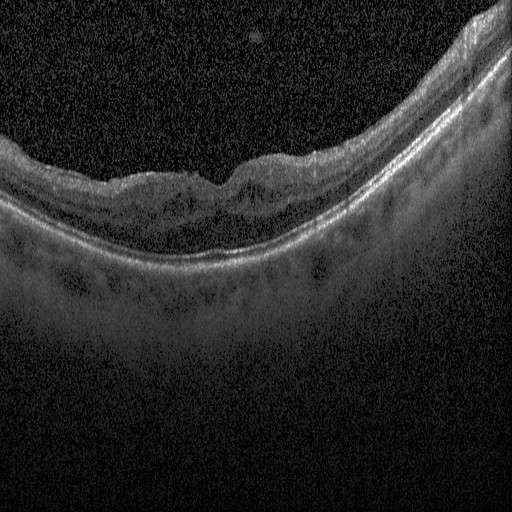 Retinal OCT B-scan, horizontal scan through the fovea, spectral-domain OCT, Heidelberg Spectralis OCT system
Diagnosis: diabetic macular edema (DME).